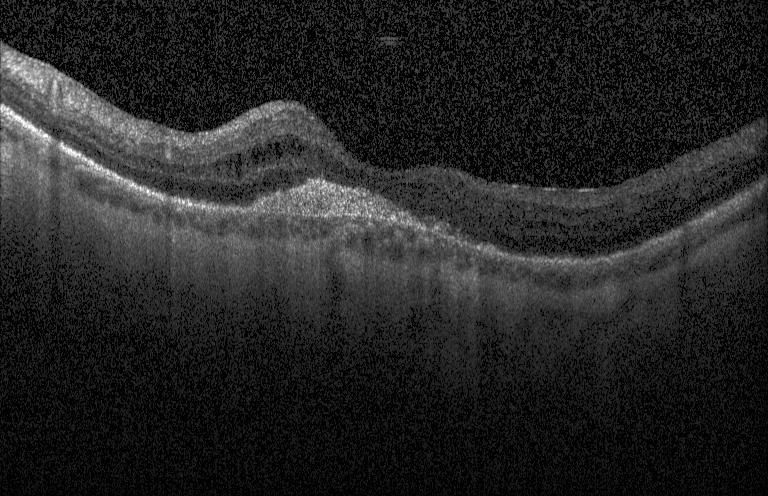 Retinal OCT cross-section.
Diagnosis: choroidal neovascularization (CNV).